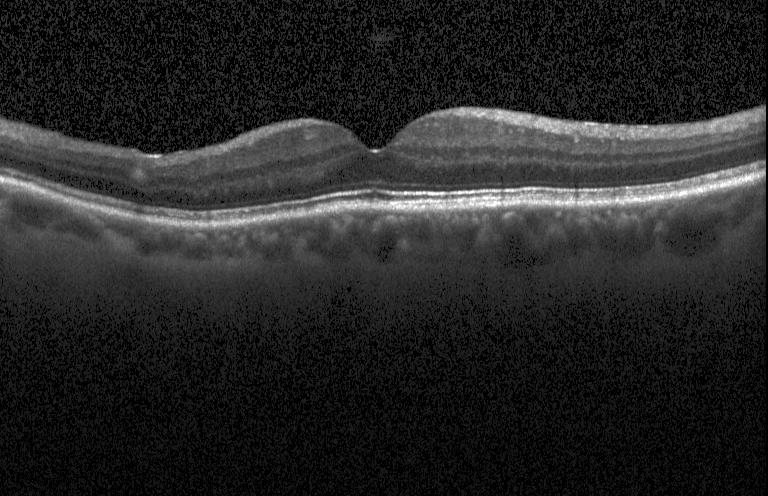
OCT finding: no choroidal neovascularization, no diabetic macular edema, and no drusen.